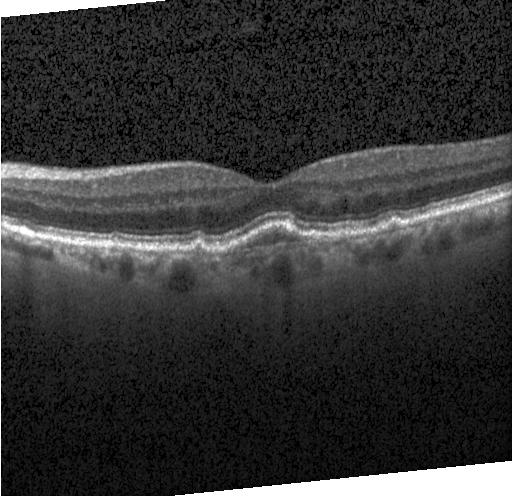 OCT B-scan showing choroidal neovascularization (CNV).